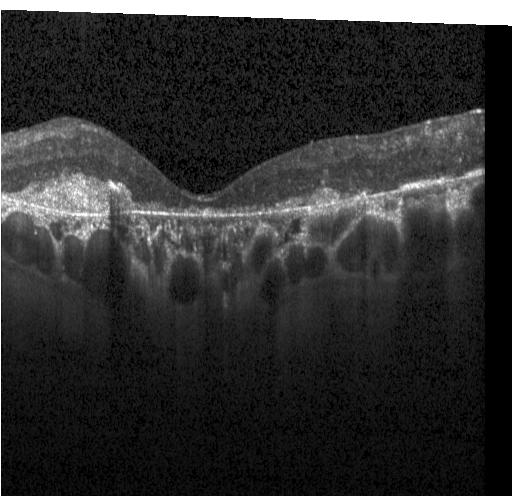
Retinal OCT cross-section, Heidelberg Spectralis
Finding: choroidal neovascularization.